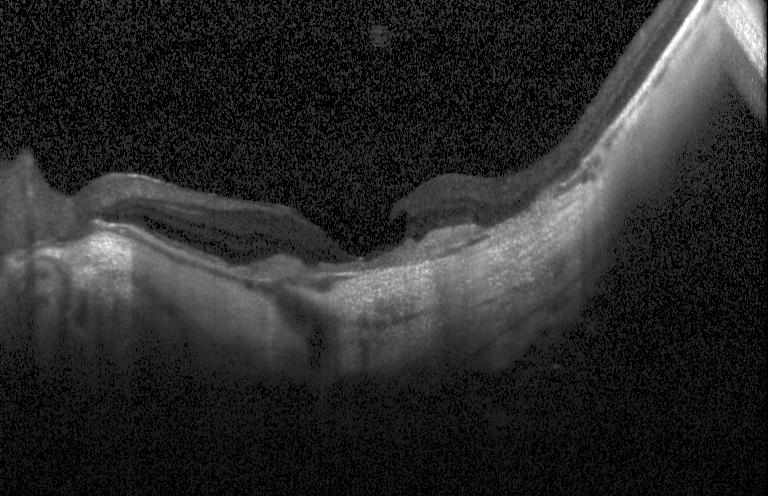

Optical coherence tomography scan · fovea-centered · spectral-domain OCT
Finding: a choroidal neovascular membrane.